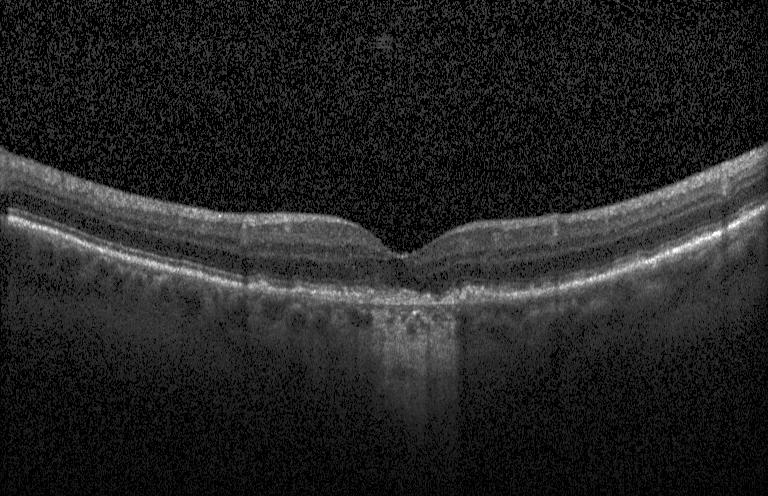

Diagnosis: choroidal neovascularization (CNV).